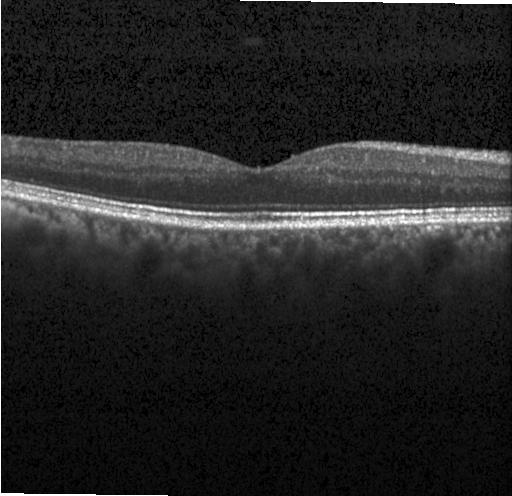

OCT scan showing no CNV, no DME, and no drusen.